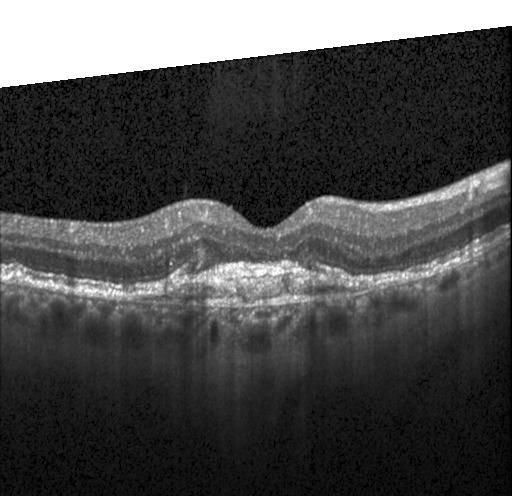
Spectral-domain OCT · optical coherence tomography scan. Impression: a choroidal neovascular membrane.